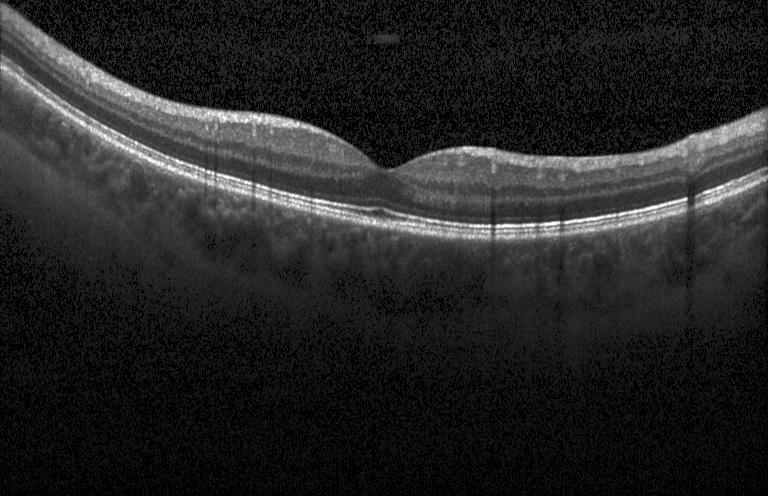

Assessment: no CNV, no DME, and no drusen.